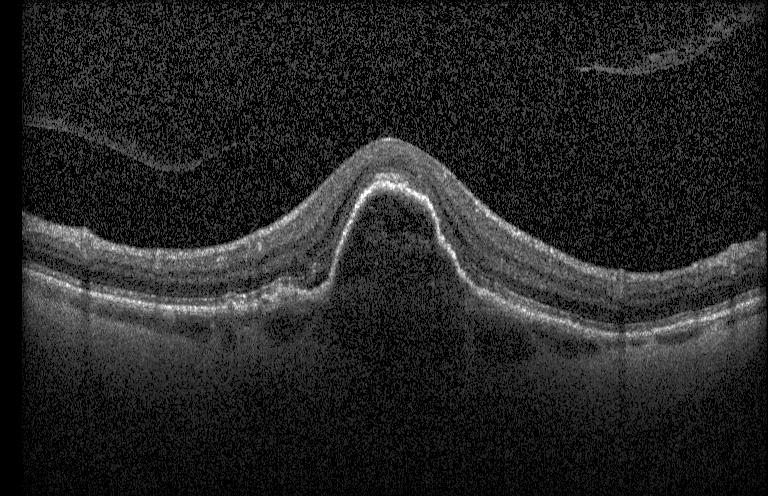 OCT finding: a choroidal neovascular membrane.